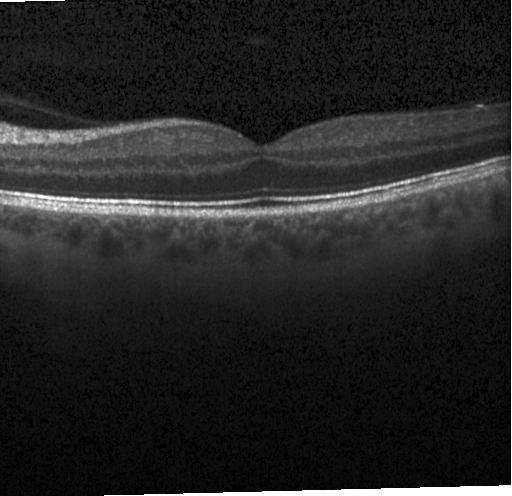 OCT finding: no choroidal neovascularization, diabetic macular edema, or drusen.